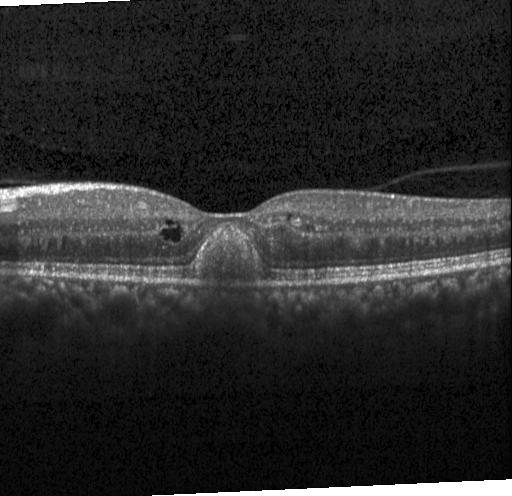

Diagnosis: a choroidal neovascular membrane.